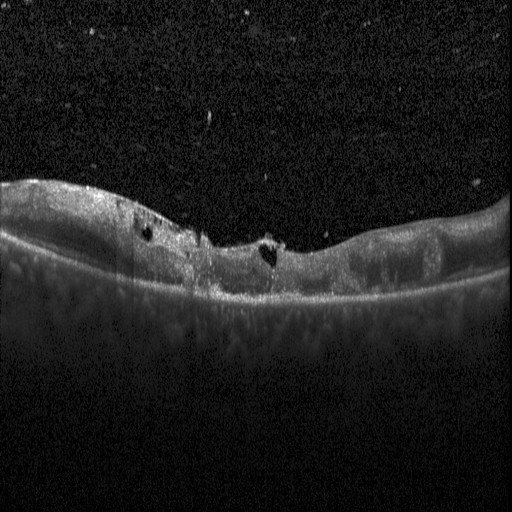 Macular scan · SD-OCT · retinal OCT cross-section
Impression: diabetic macular edema.